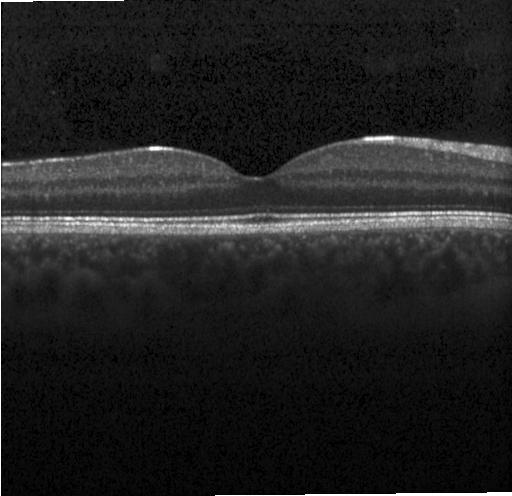
Optical coherence tomography B-scan. Heidelberg Spectralis OCT system
This B-scan demonstrates no evidence of choroidal neovascularization, diabetic macular edema, or drusen.